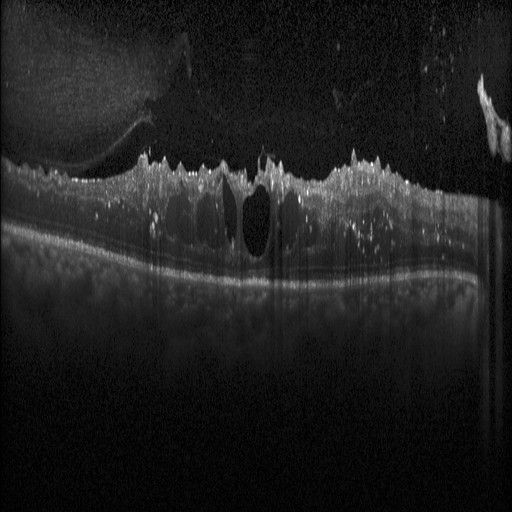 Optical coherence tomography B-scan, acquired on a Heidelberg Spectralis, spectral-domain OCT. This B-scan demonstrates diabetic macular edema.